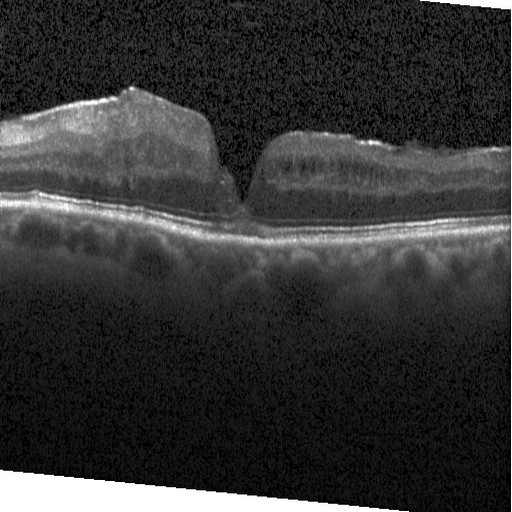

OCT B-scan; through the macula; acquired on a Heidelberg Spectralis — The scan shows diabetic macular edema.